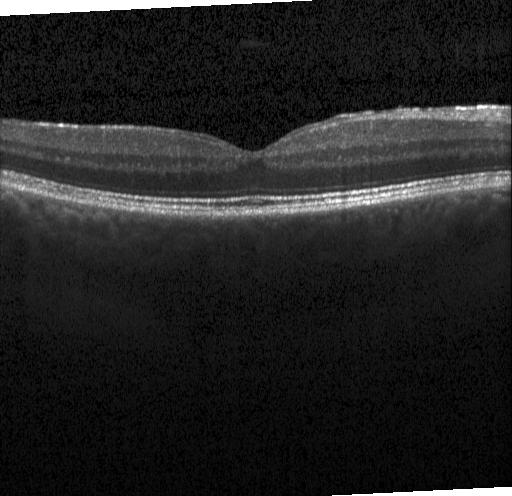 Macular scan · spectral-domain optical coherence tomography · retinal OCT cross-section · acquired on a Heidelberg Spectralis
Assessment: no evidence of CNV, DME, or drusen.